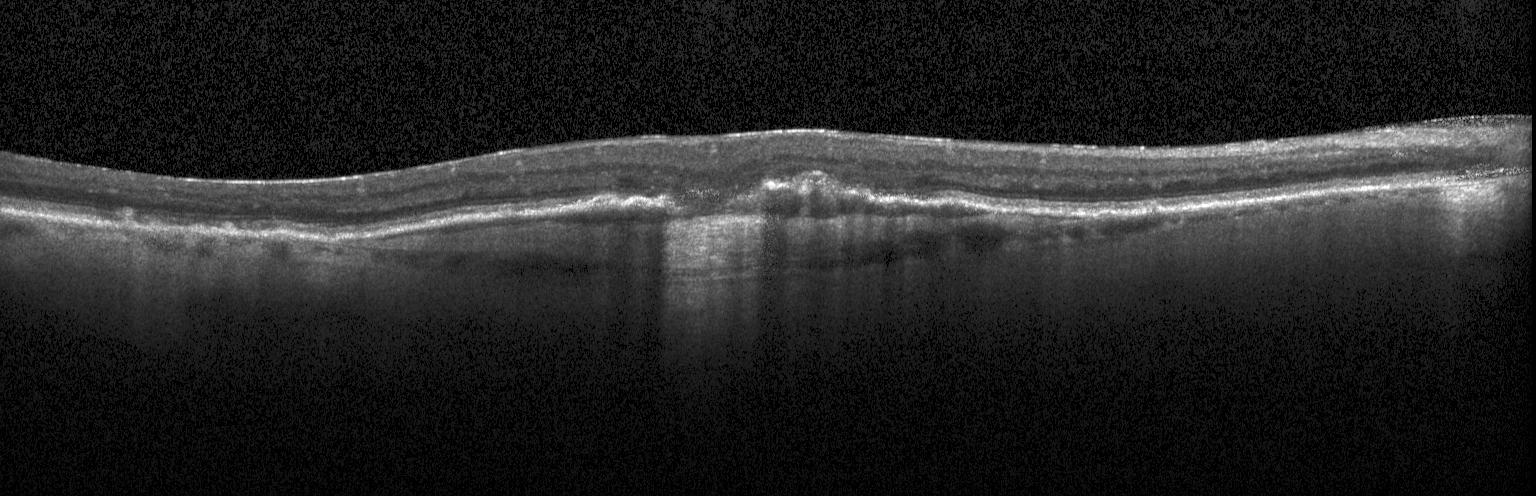
Optical coherence tomography B-scan.
Macular OCT: choroidal neovascularization.